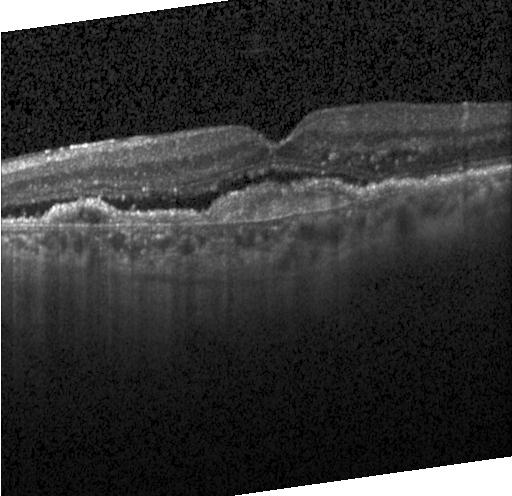 OCT B-scan showing CNV.